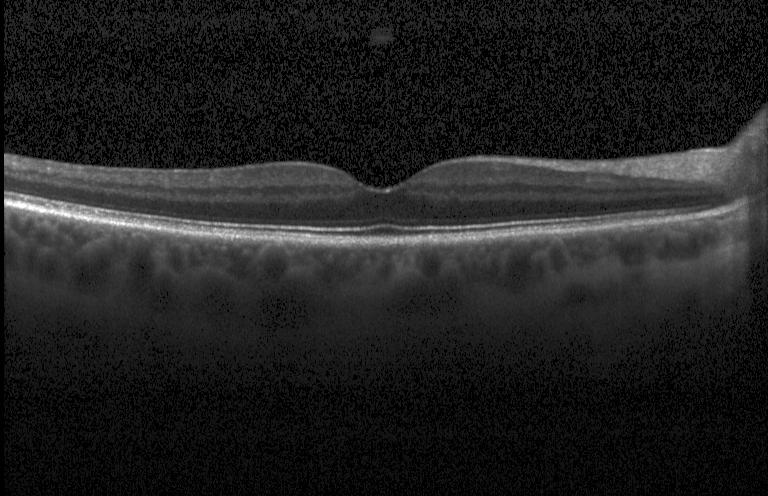 Finding: neither CNV, DME, nor drusen.